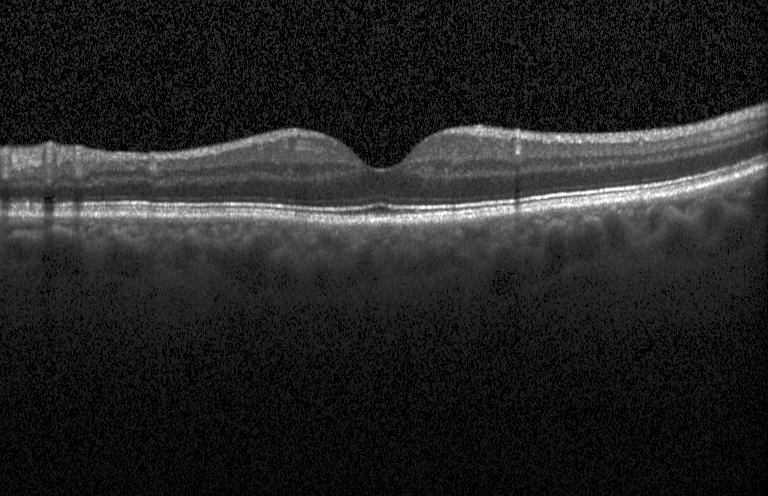 OCT line scan · acquired on a Heidelberg Spectralis.
Impression: no choroidal neovascularization, diabetic macular edema, or drusen.